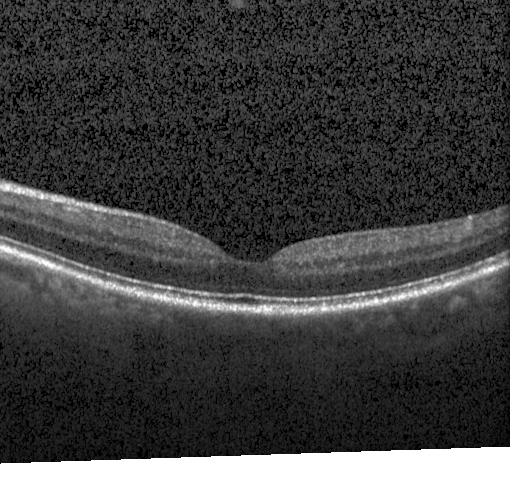
Spectral-domain OCT, macular scan, acquired on a Heidelberg Spectralis, optical coherence tomography B-scan. This B-scan demonstrates no choroidal neovascularization, diabetic macular edema, or drusen.